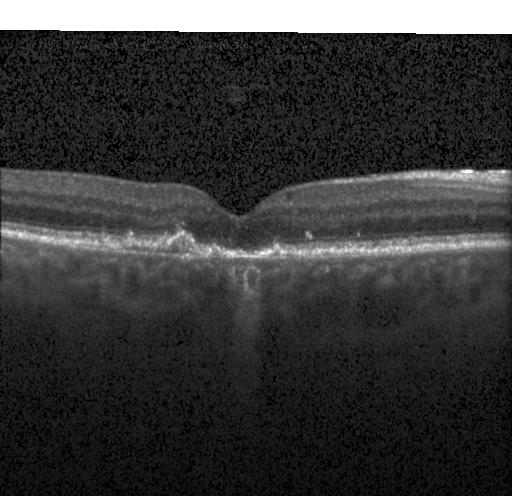
Retinal OCT cross-section showing a choroidal neovascular membrane.